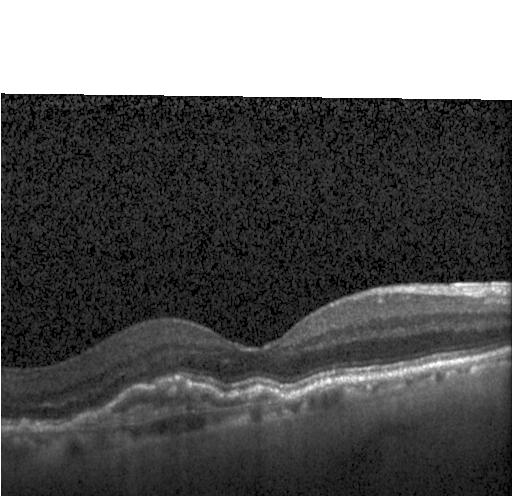
Instrument: Heidelberg Spectralis · macular scan · retinal OCT cross-section. Dx: a choroidal neovascular membrane.